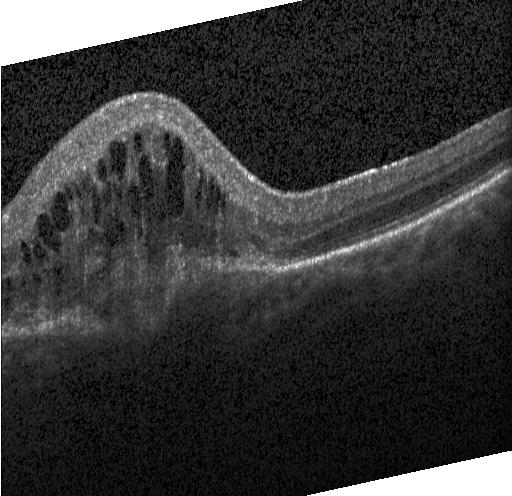
Horizontal scan through the fovea. SD-OCT. Optical coherence tomography B-scan. Acquired on a Heidelberg Spectralis.
Diagnosis: a choroidal neovascular membrane.